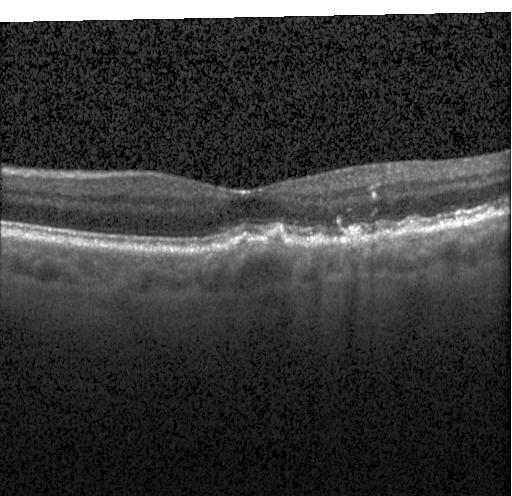 OCT finding: drusen.